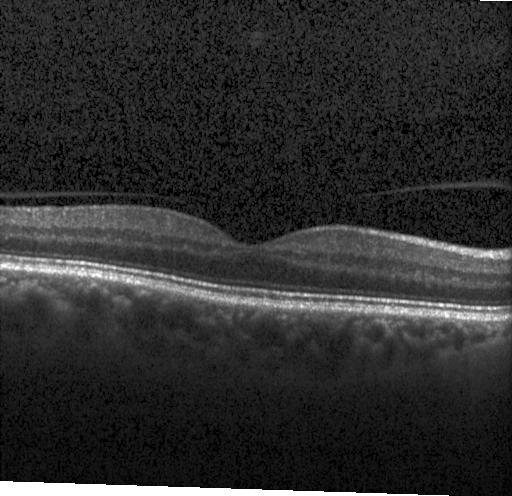 Diagnosis: no CNV, no DME, and no drusen.